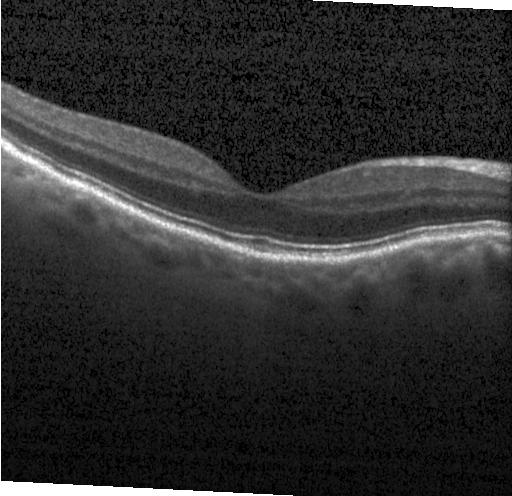

Heidelberg Spectralis OCT system; through the macula; OCT line scan; spectral-domain optical coherence tomography.
Dx: no choroidal neovascularization, no diabetic macular edema, and no drusen.